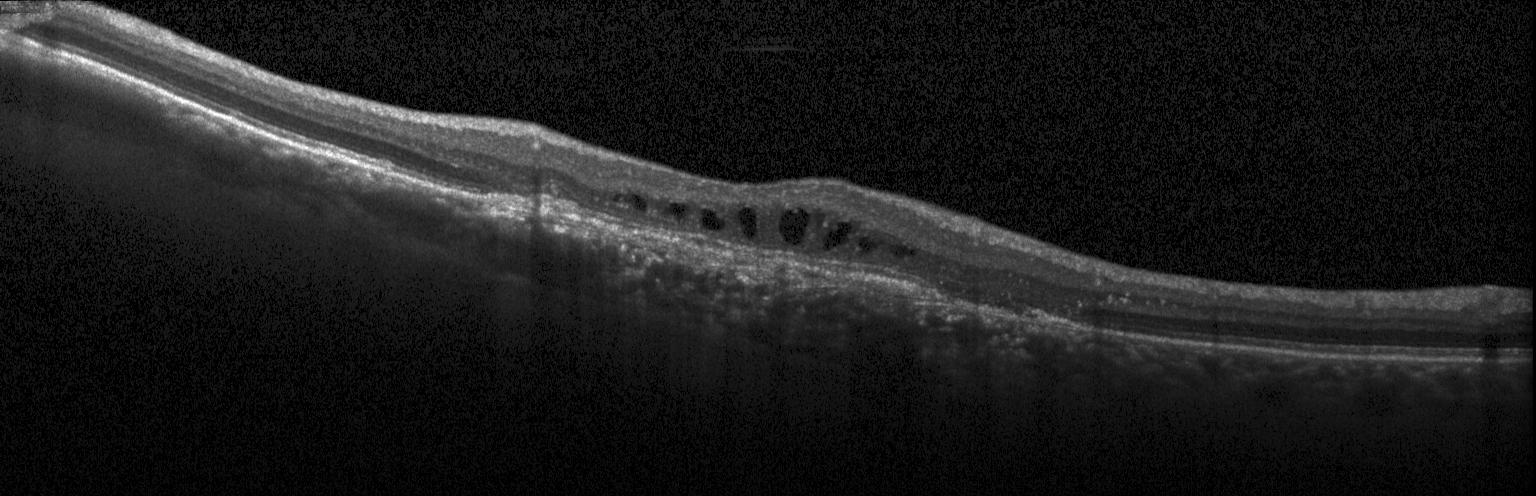 Optical coherence tomography scan. This B-scan demonstrates choroidal neovascularization (CNV).